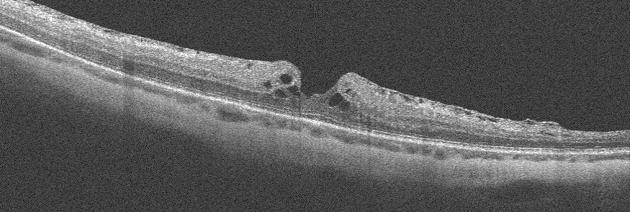

Left eye, OCT B-scan — This B-scan demonstrates vitreomacular interface disease (VID).